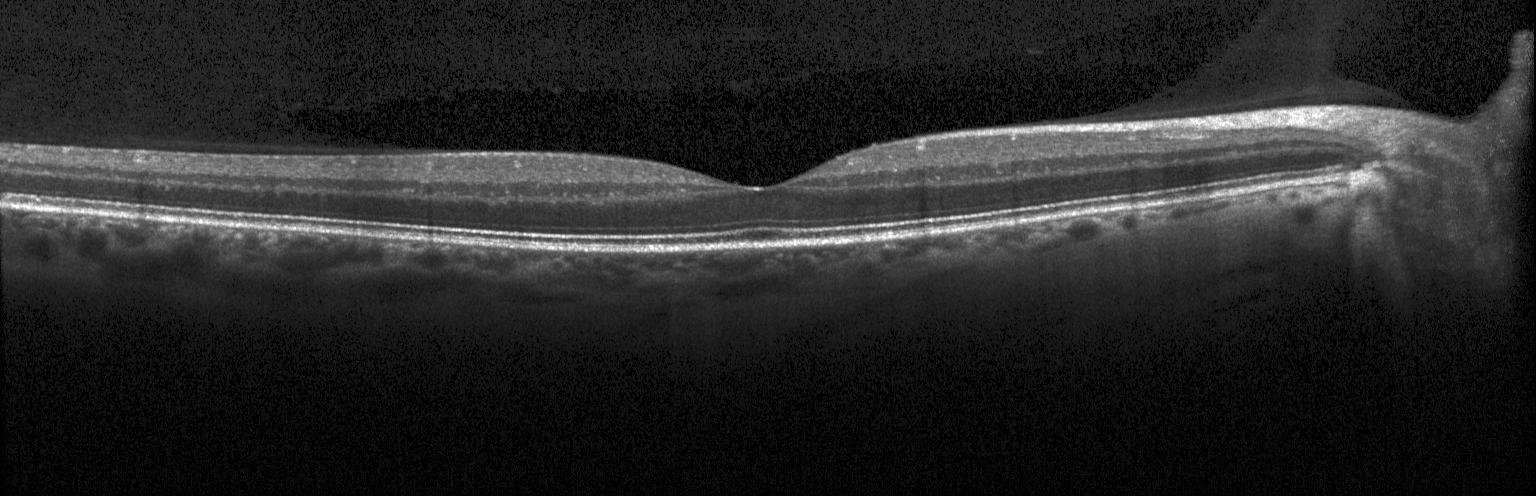

Retinal OCT cross-section · SD-OCT · centered on the fovea. Macular OCT: no CNV, DME, or drusen.